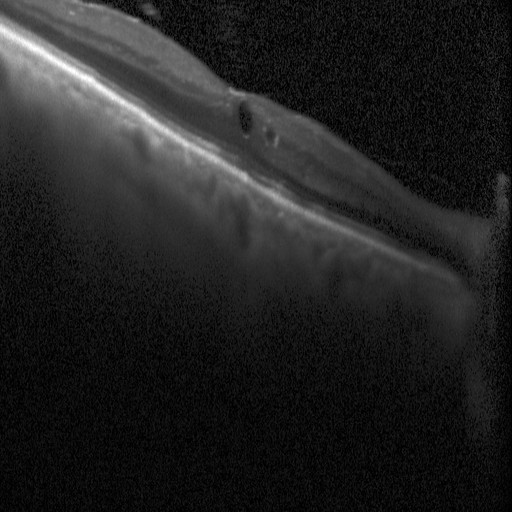

Horizontal scan through the fovea, instrument: Heidelberg Spectralis, OCT B-scan, spectral-domain optical coherence tomography.
Impression: DME.